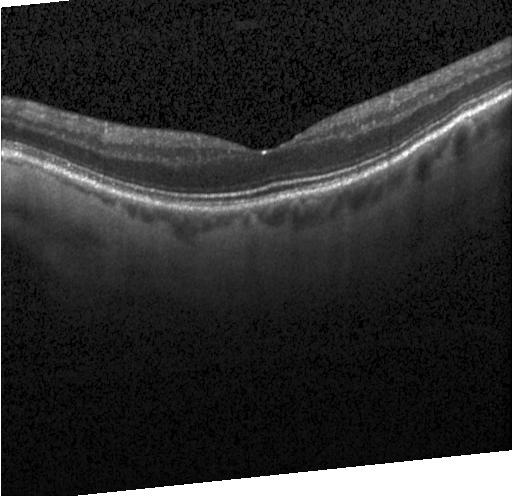

This B-scan demonstrates no evidence of choroidal neovascularization, diabetic macular edema, or drusen.